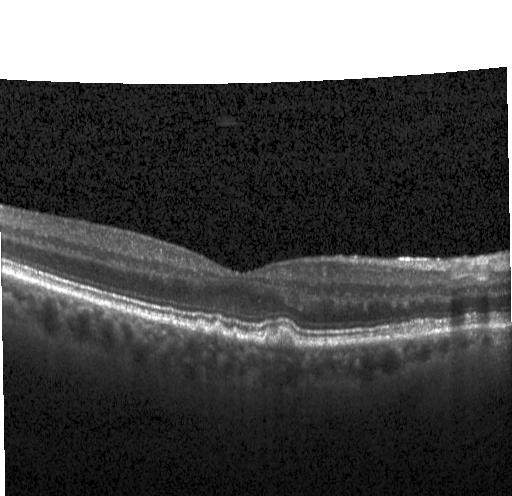

Spectral-domain OCT B-scan: multiple drusen.